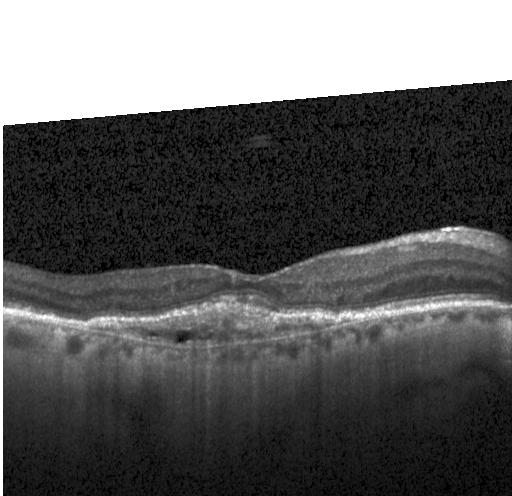
Retinal OCT cross-section
Assessment: a choroidal neovascular membrane.